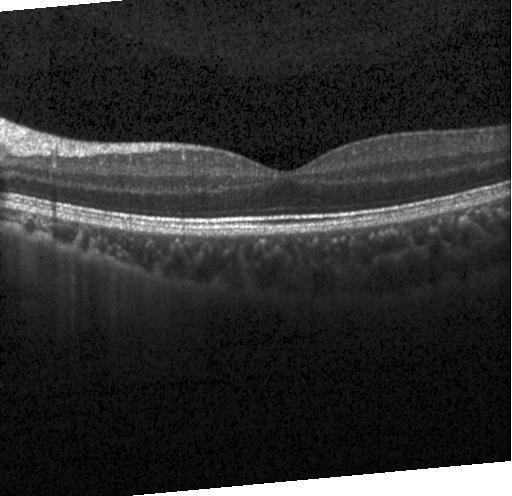 Retinal OCT cross-section. Diagnosis: no choroidal neovascularization, no diabetic macular edema, and no drusen.